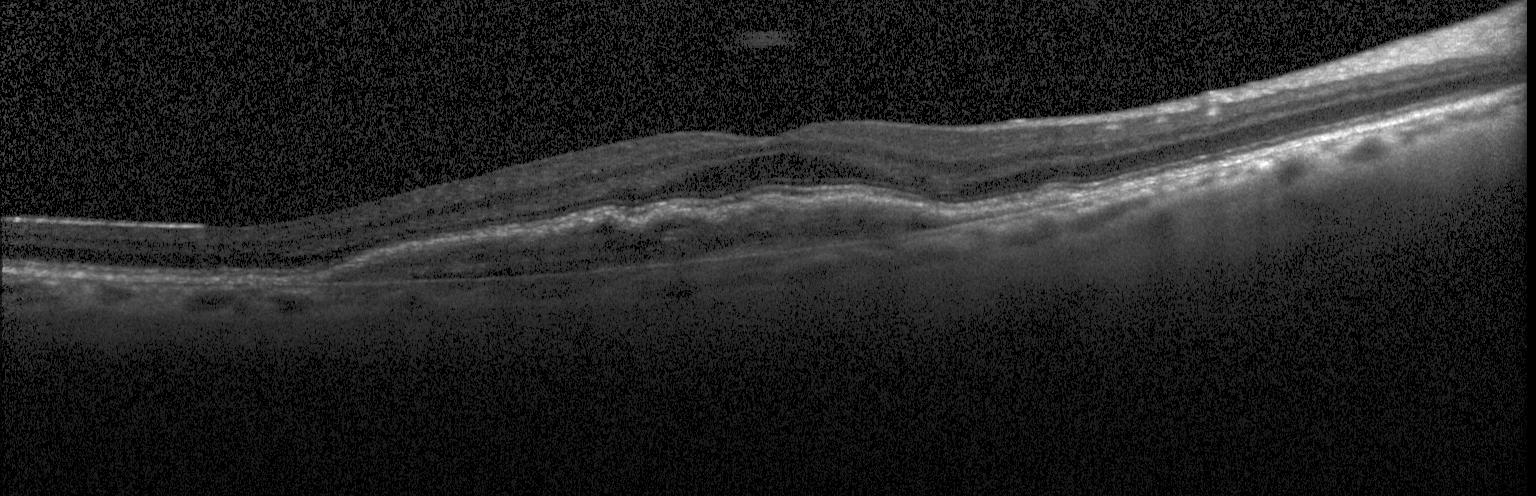 Choroidal neovascularization (CNV).